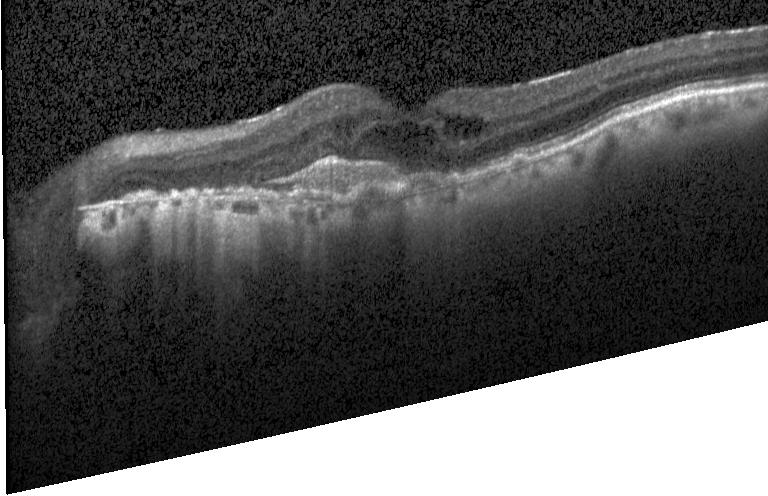
OCT B-scan showing choroidal neovascularization (CNV).